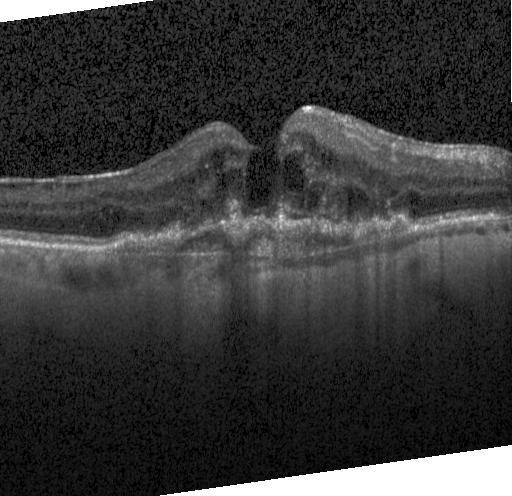
A choroidal neovascular membrane.